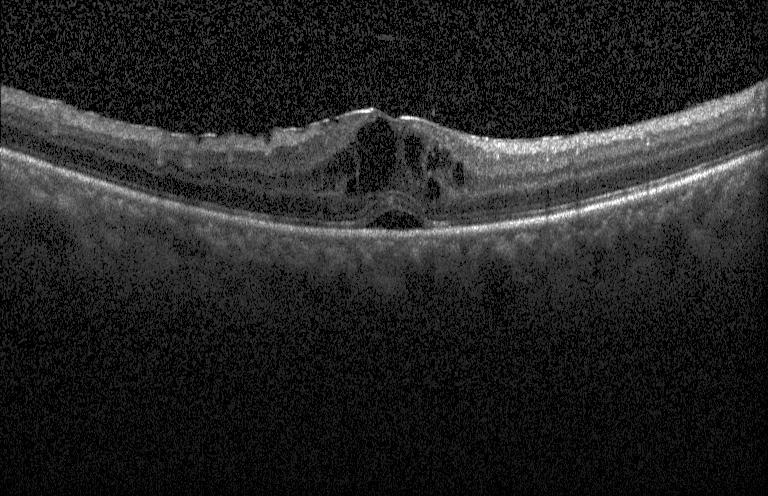

Retinal OCT cross-section — Dx: DME.